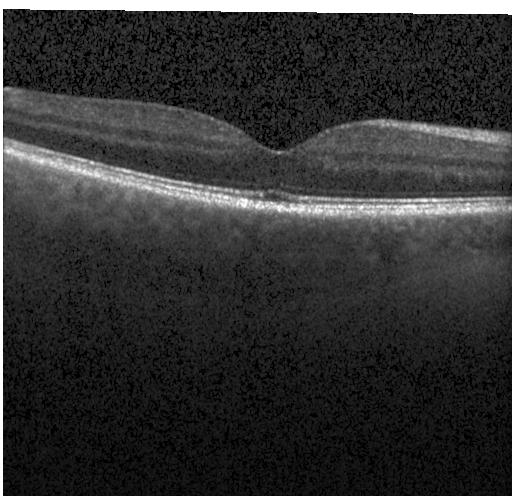

Spectral-domain OCT, macular scan, optical coherence tomography scan. Impression: no choroidal neovascularization, no diabetic macular edema, and no drusen.